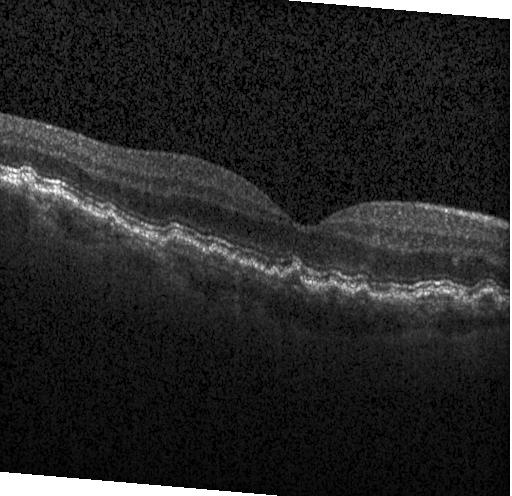 Spectral-domain OCT; retinal OCT B-scan — Macular OCT: sub-RPE drusenoid deposits.